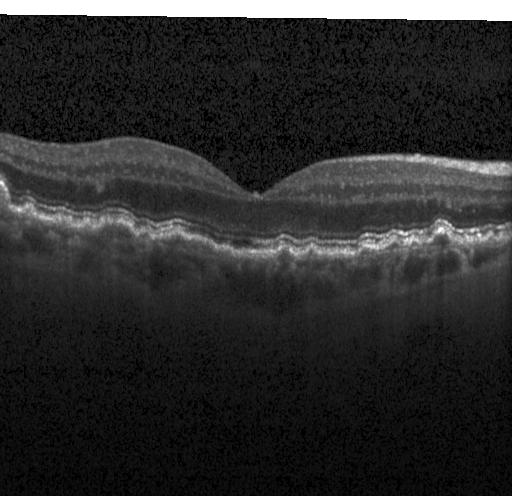
Optical coherence tomography scan.
Impression: drusen.